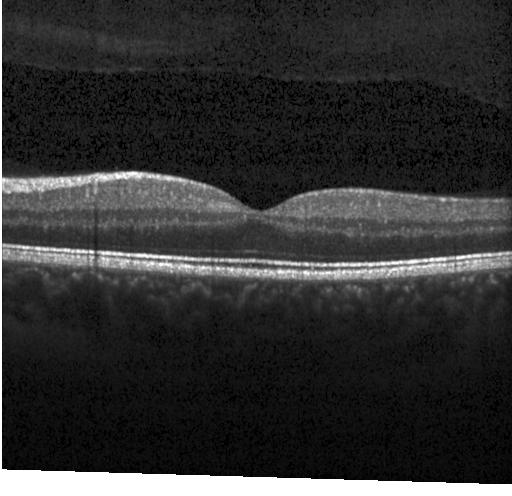
Spectral-domain OCT; instrument: Heidelberg Spectralis; centered on the fovea; optical coherence tomography B-scan — The scan shows no evidence of choroidal neovascularization, diabetic macular edema, or drusen.